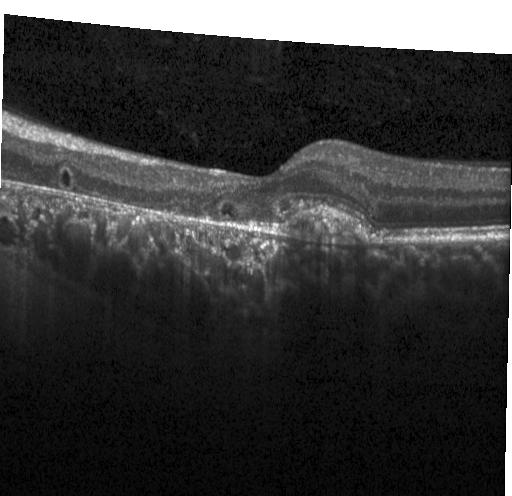 Impression: choroidal neovascularization.